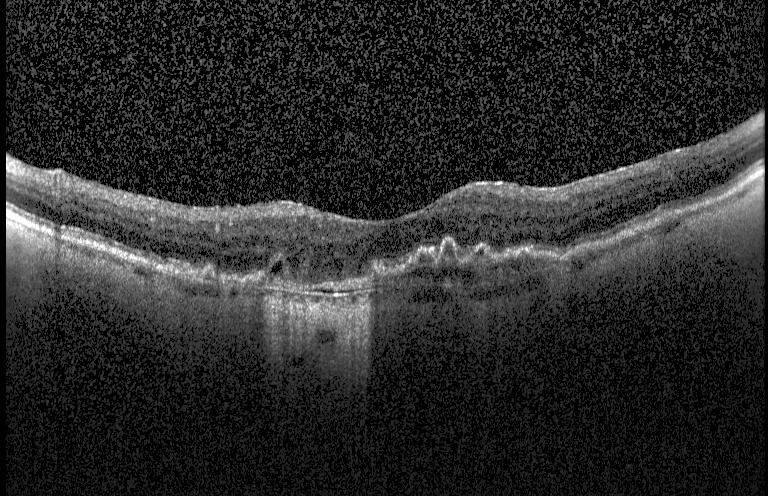 Retinal OCT B-scan, acquired on a Heidelberg Spectralis
Macular OCT: choroidal neovascularization (CNV).